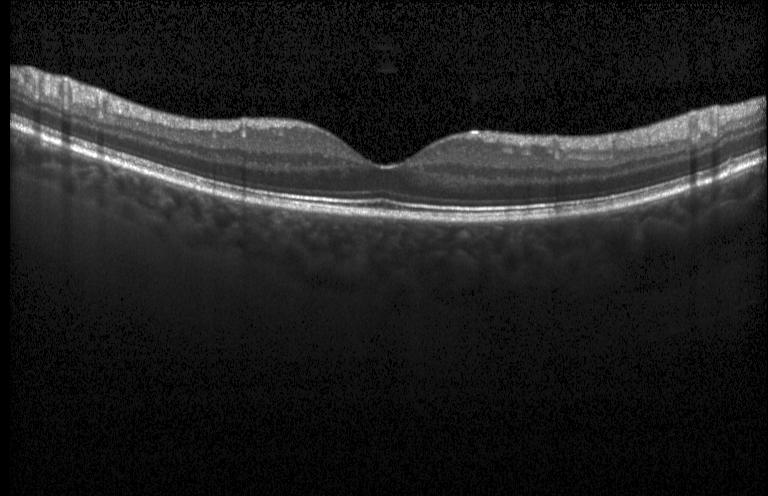

This B-scan demonstrates no choroidal neovascularization, diabetic macular edema, or drusen.